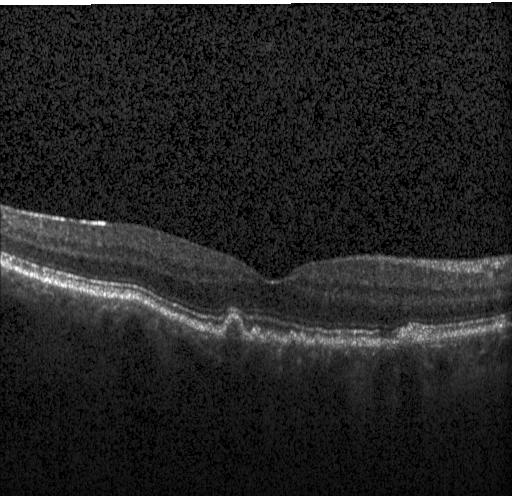

Retinal OCT B-scan — OCT finding: drusen.